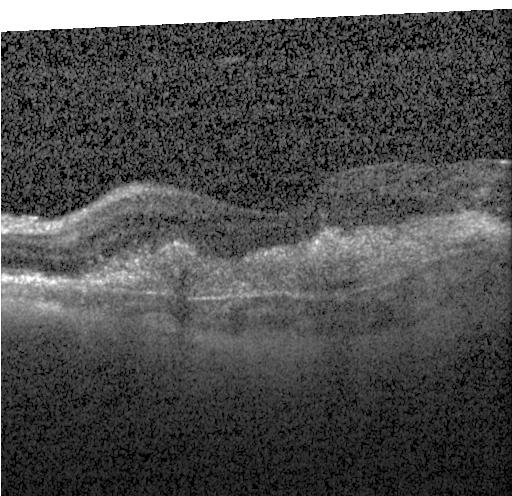 Retinal OCT cross-section. Impression: a choroidal neovascular membrane.